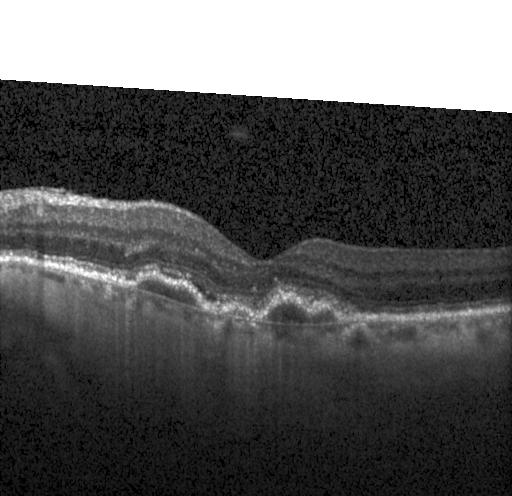

Horizontal scan through the fovea, retinal OCT cross-section, instrument: Heidelberg Spectralis
Diagnosis: CNV.